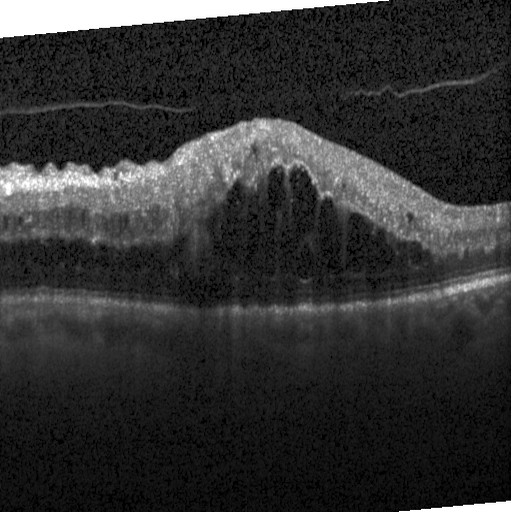

Finding: DME.